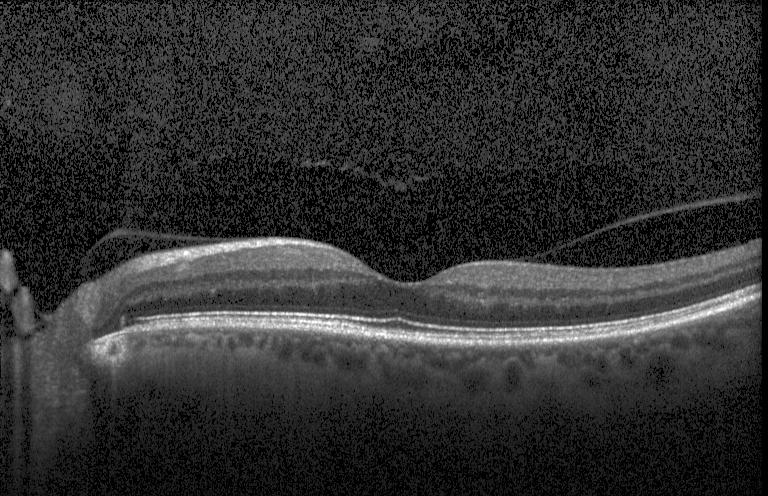 Optical coherence tomography scan · instrument: Heidelberg Spectralis · fovea-centered.
The scan shows no evidence of choroidal neovascularization, diabetic macular edema, or drusen.